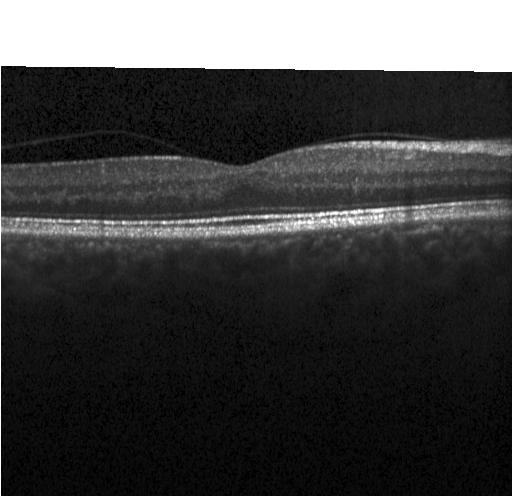 Retinal OCT cross-section showing neither CNV, DME, nor drusen.